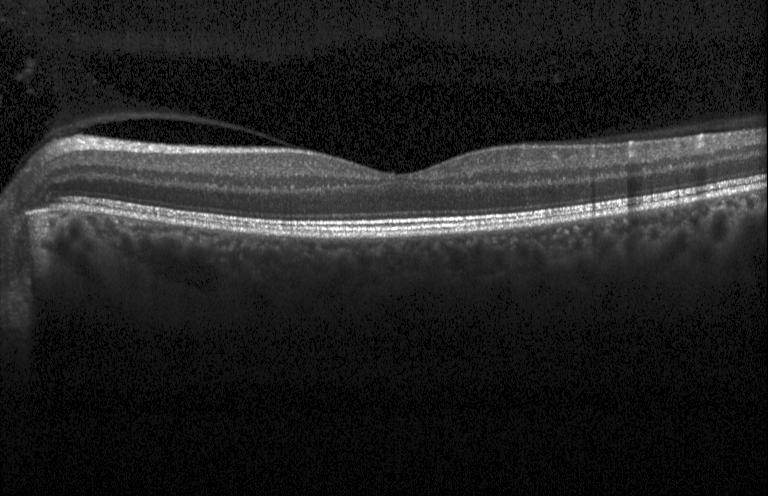
Diagnosis: neither choroidal neovascularization, diabetic macular edema, nor drusen.